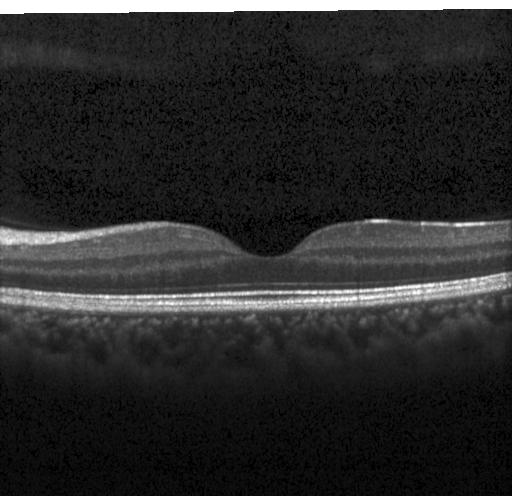
Retinal OCT B-scan. Fovea-centered — Assessment: no choroidal neovascularization, no diabetic macular edema, and no drusen.